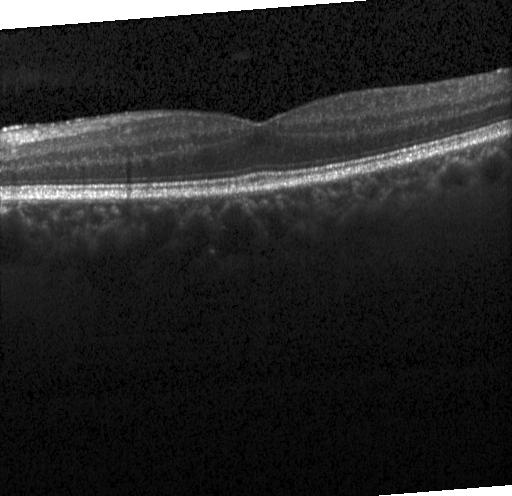
OCT line scan, SD-OCT, Heidelberg Spectralis — OCT finding: no choroidal neovascularization, diabetic macular edema, or drusen.